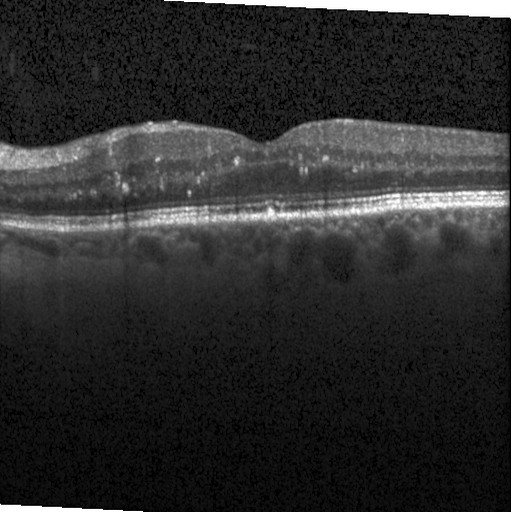

Optical coherence tomography B-scan
Assessment: diabetic macular edema (DME).